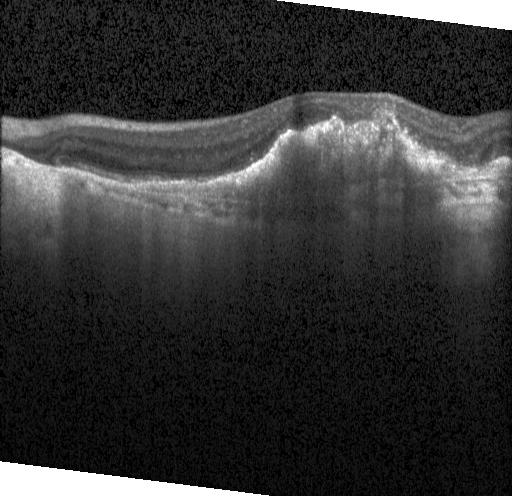 Spectral-domain optical coherence tomography; optical coherence tomography B-scan — Diagnosis: choroidal neovascularization.